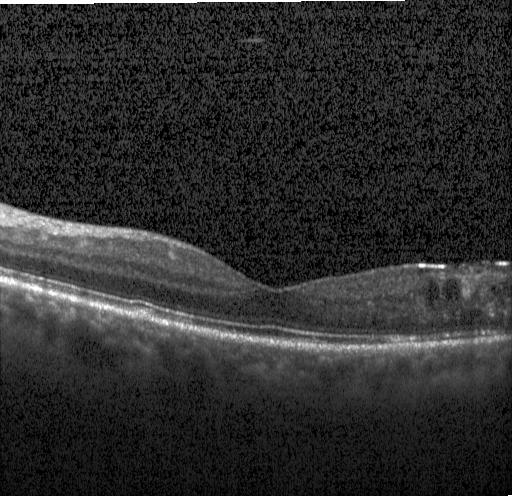
SD-OCT, horizontal scan through the fovea, optical coherence tomography scan, instrument: Heidelberg Spectralis.
Diagnosis: diabetic macular edema (DME).